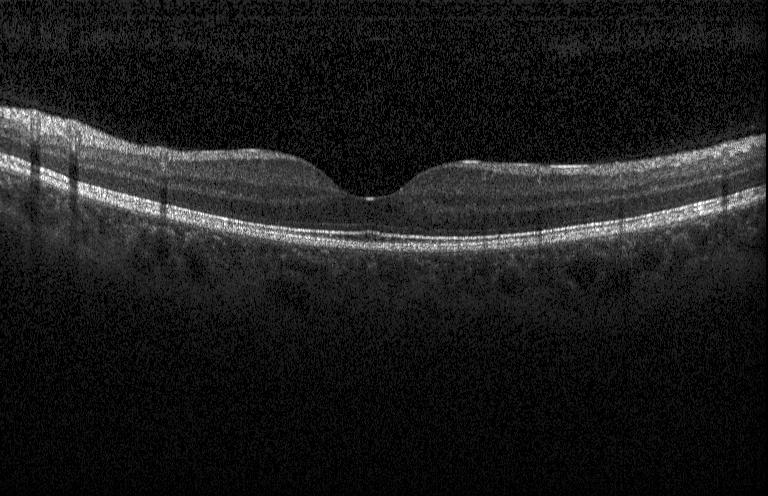

SD-OCT · acquired on a Heidelberg Spectralis · OCT B-scan · centered on the fovea.
Dx: no evidence of CNV, DME, or drusen.